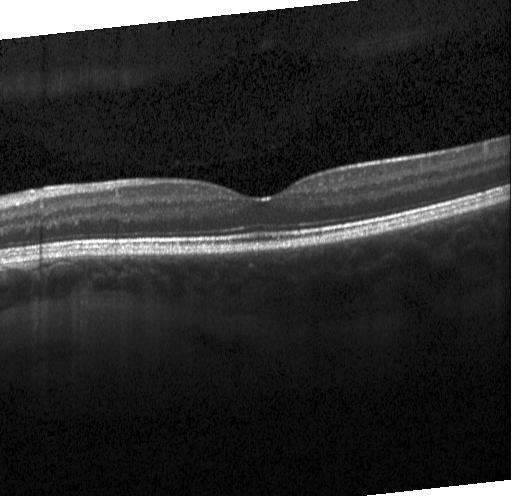
Retinal OCT cross-section.
The scan shows no CNV, DME, or drusen.